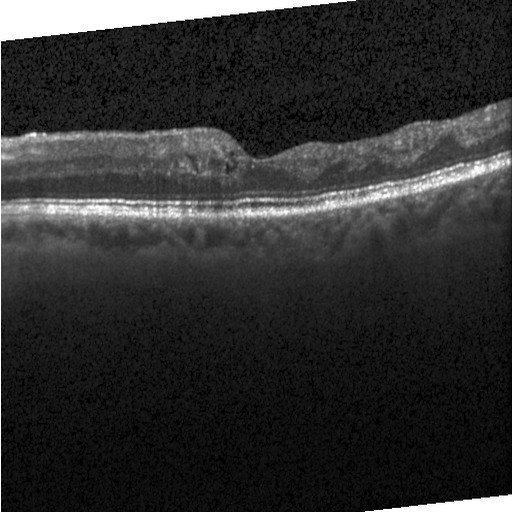
Dx: DME.